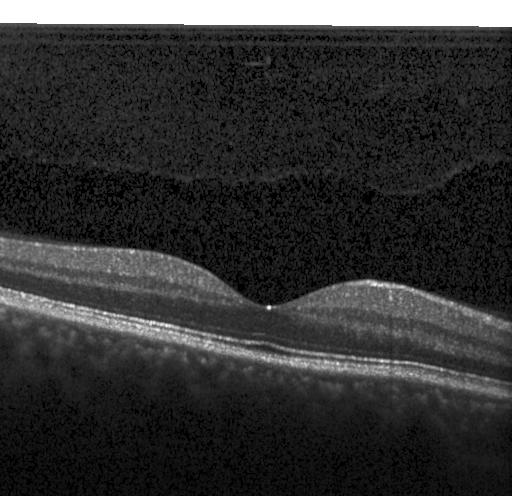 This B-scan demonstrates neither choroidal neovascularization, diabetic macular edema, nor drusen.